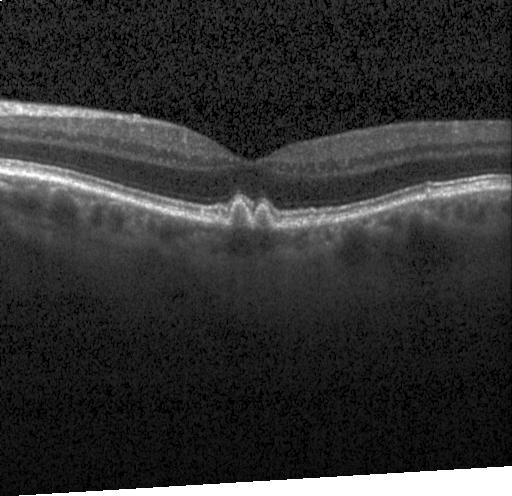
Macular OCT demonstrating multiple drusen.